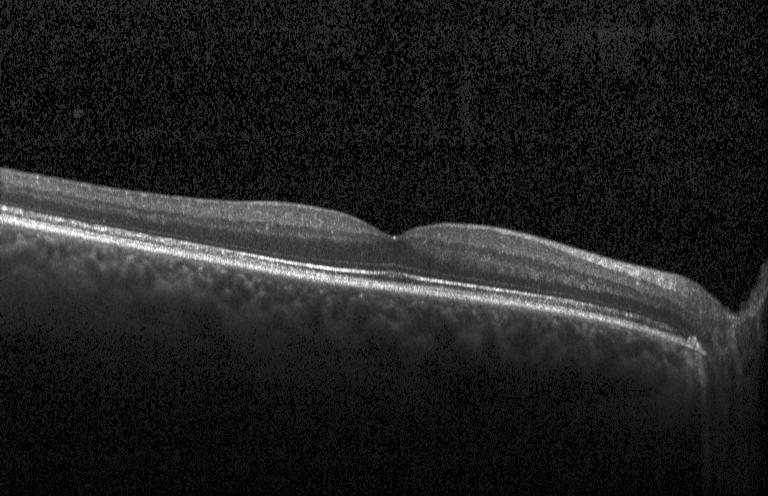 Acquired on a Heidelberg Spectralis, OCT B-scan
This B-scan demonstrates no choroidal neovascularization, no diabetic macular edema, and no drusen.